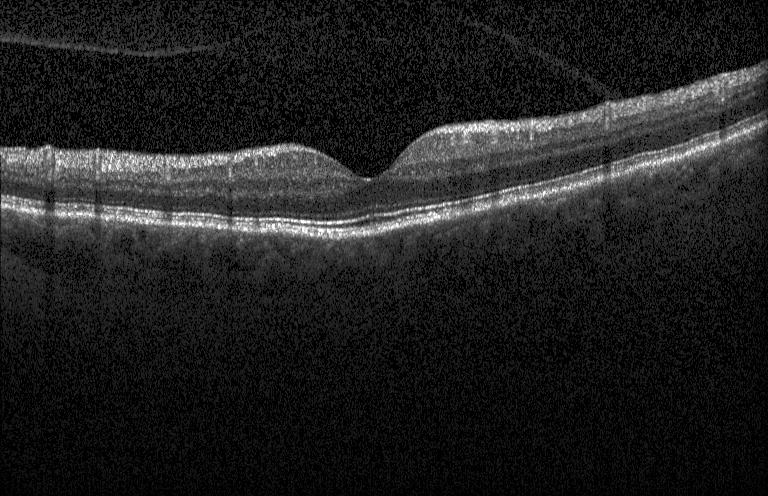 Diagnosis: neither choroidal neovascularization, diabetic macular edema, nor drusen.